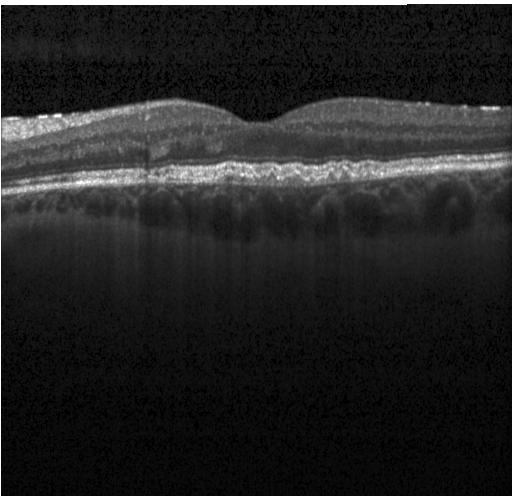 Retinal OCT B-scan
Finding: drusen.